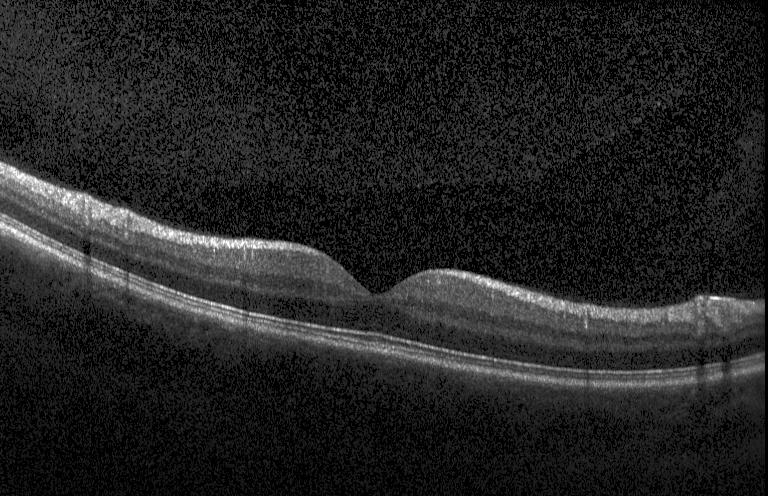
Heidelberg Spectralis OCT system. Spectral-domain optical coherence tomography. Optical coherence tomography scan — The scan shows neither choroidal neovascularization, diabetic macular edema, nor drusen.